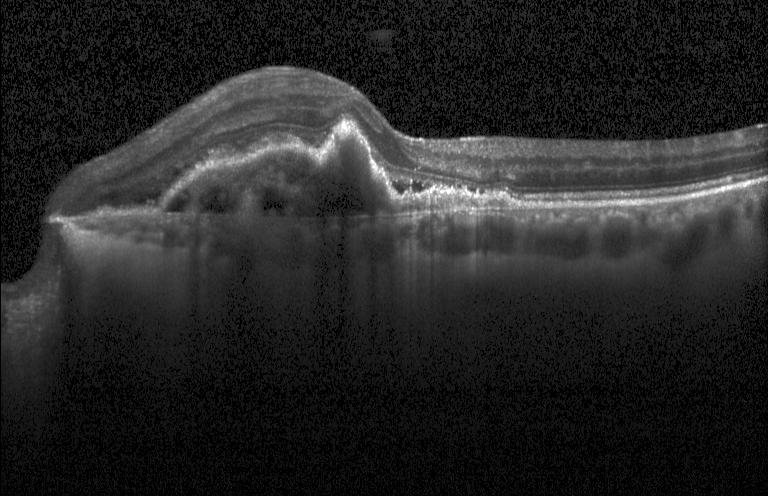

Retinal OCT cross-section showing a choroidal neovascular membrane.